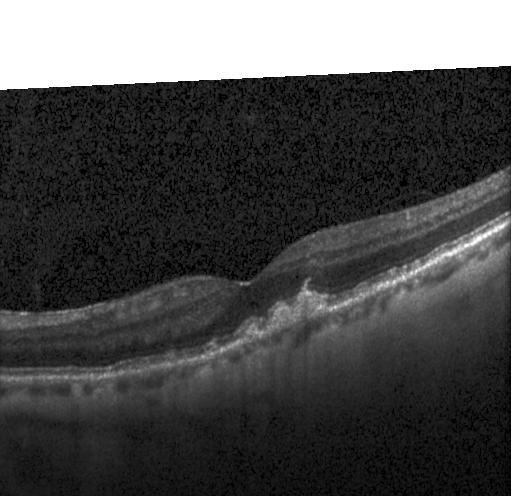

OCT B-scan — Impression: drusen.